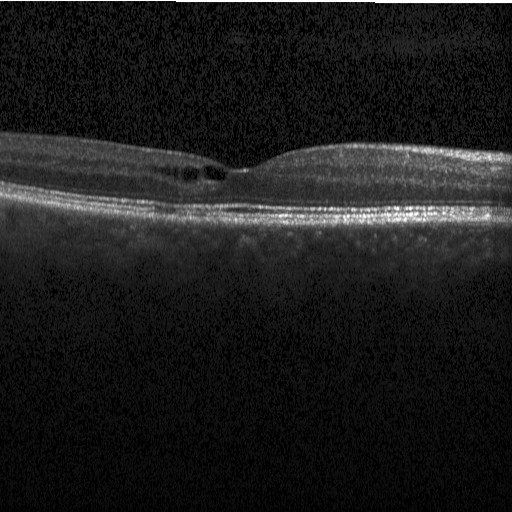

Spectral-domain OCT, optical coherence tomography scan — Diabetic macular edema.